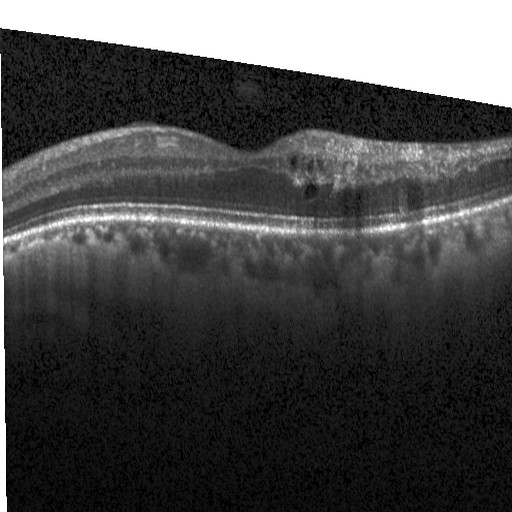

Retinal OCT cross-section · through the macula
Impression: diabetic macular edema (DME).